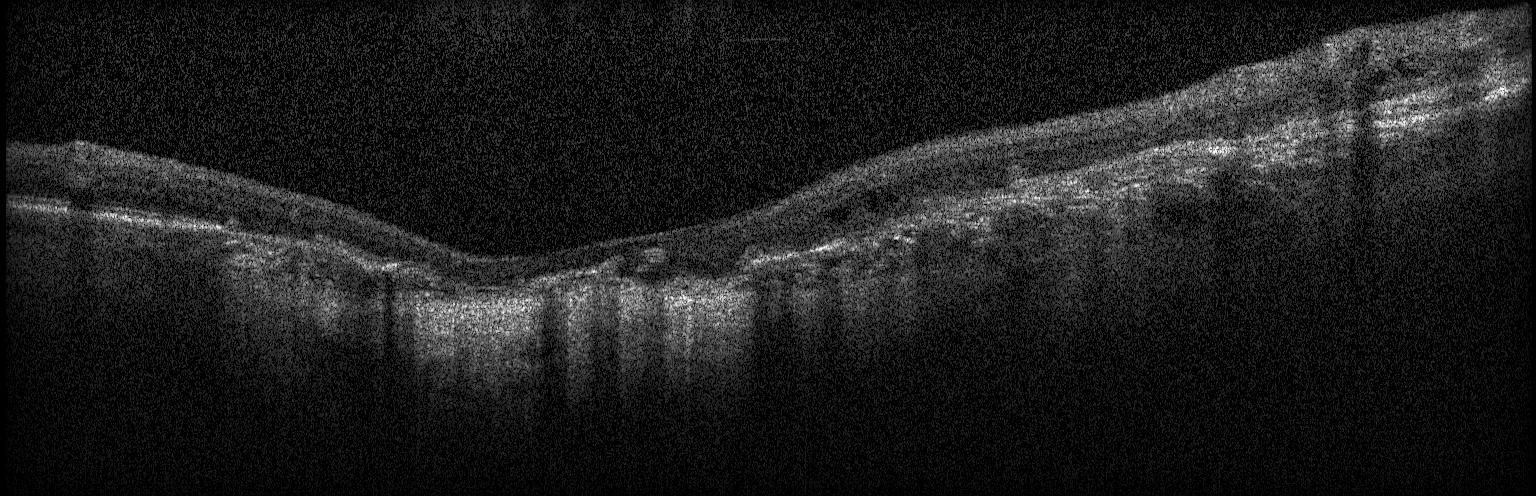
Heidelberg Spectralis · centered on the fovea · spectral-domain optical coherence tomography · retinal OCT cross-section. Assessment: choroidal neovascularization.